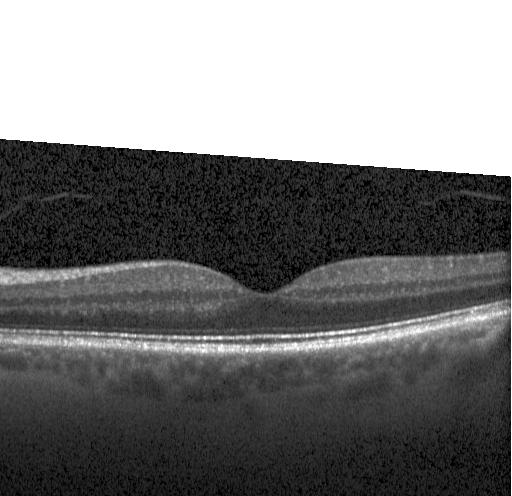
Assessment: no choroidal neovascularization, diabetic macular edema, or drusen.